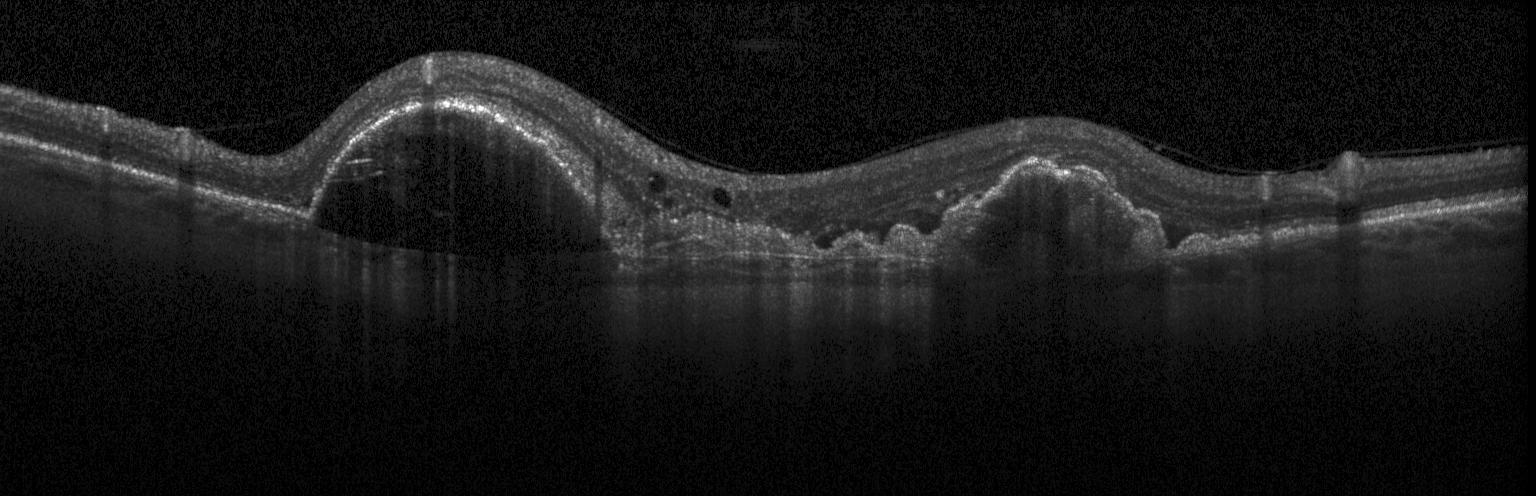 Retinal OCT B-scan.
Finding: choroidal neovascularization (CNV).